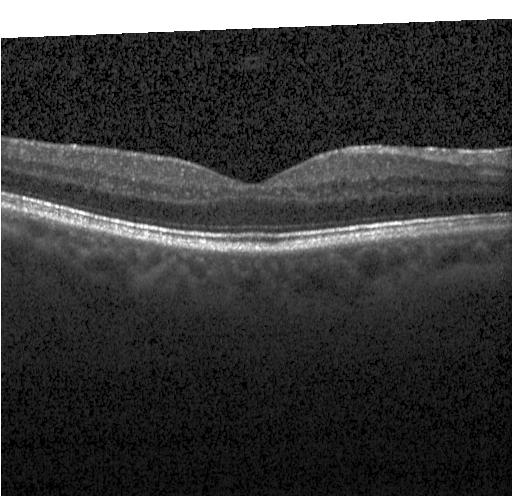

Assessment: no choroidal neovascularization, diabetic macular edema, or drusen.